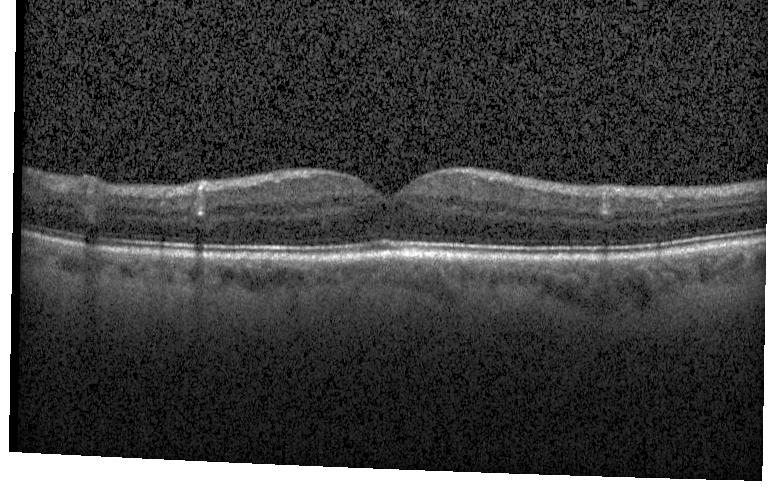 Diagnosis: no evidence of choroidal neovascularization, diabetic macular edema, or drusen.